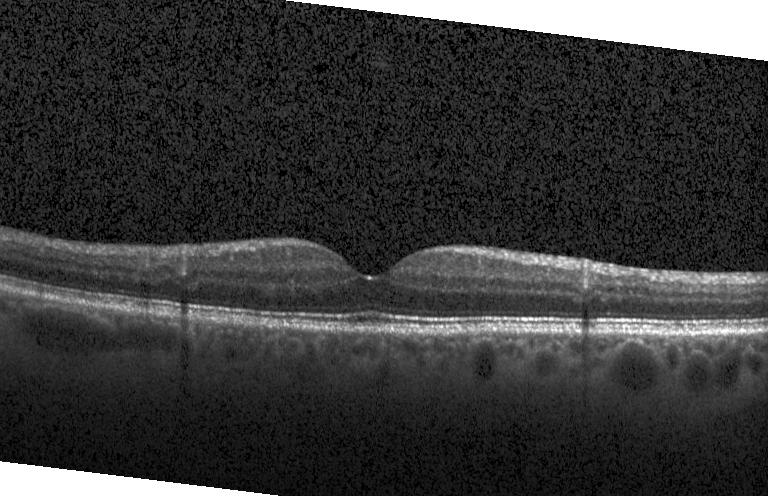
Macular OCT: no choroidal neovascularization, no diabetic macular edema, and no drusen.